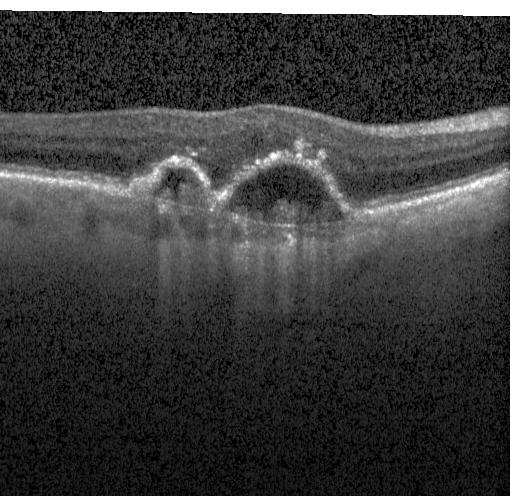

Finding: choroidal neovascularization (CNV).